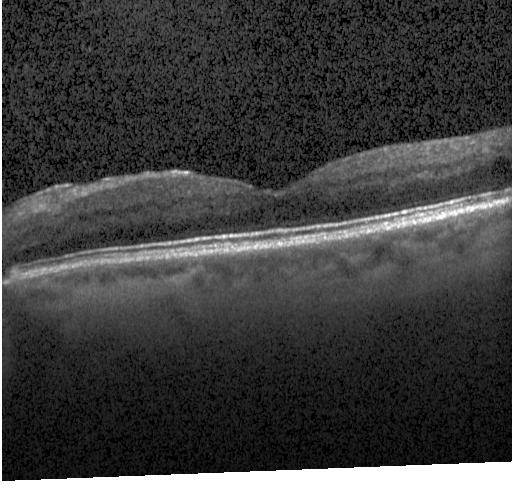

Macular OCT demonstrating no choroidal neovascularization, diabetic macular edema, or drusen.